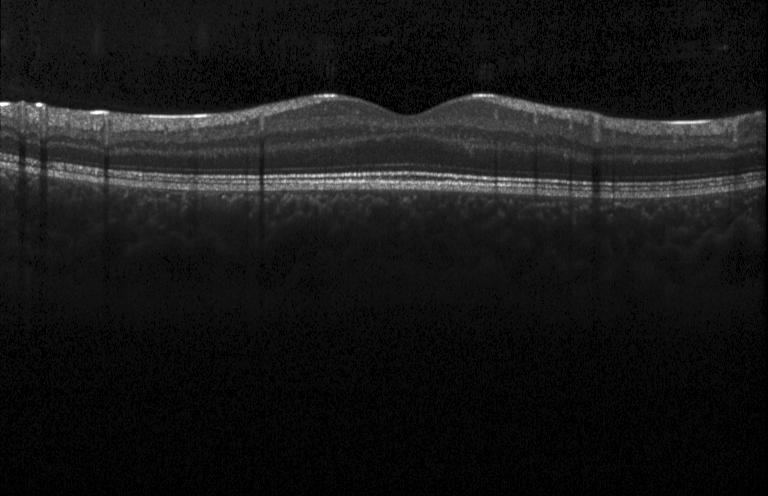 Macular OCT: no evidence of choroidal neovascularization, diabetic macular edema, or drusen.